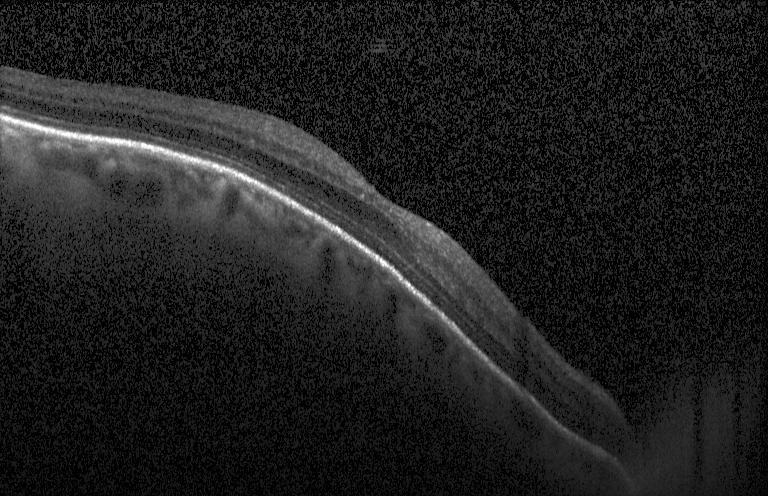

Spectral-domain OCT B-scan: no evidence of CNV, DME, or drusen.